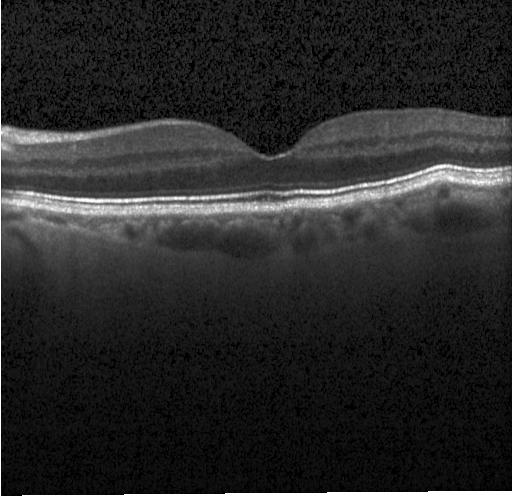

Optical coherence tomography B-scan. Instrument: Heidelberg Spectralis. Through the macula. Spectral-domain optical coherence tomography.
Dx: no CNV, no DME, and no drusen.